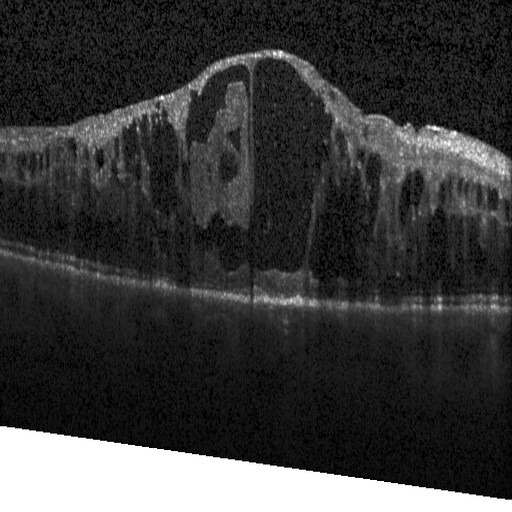 Horizontal scan through the fovea, acquired on a Heidelberg Spectralis, optical coherence tomography B-scan. Diagnosis: diabetic macular edema (DME).